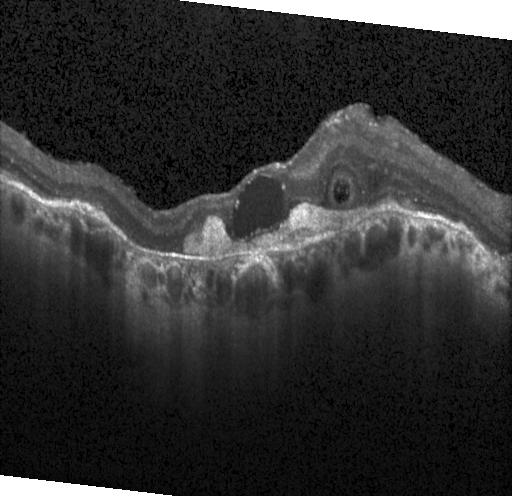
Centered on the fovea · optical coherence tomography B-scan · spectral-domain OCT.
This B-scan demonstrates a choroidal neovascular membrane.